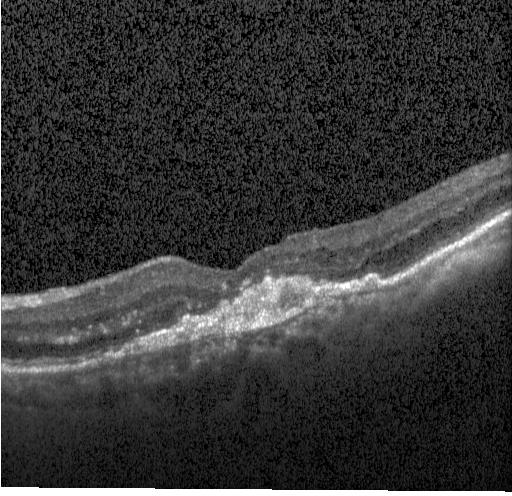
Heidelberg Spectralis · optical coherence tomography B-scan · SD-OCT
Finding: choroidal neovascularization.